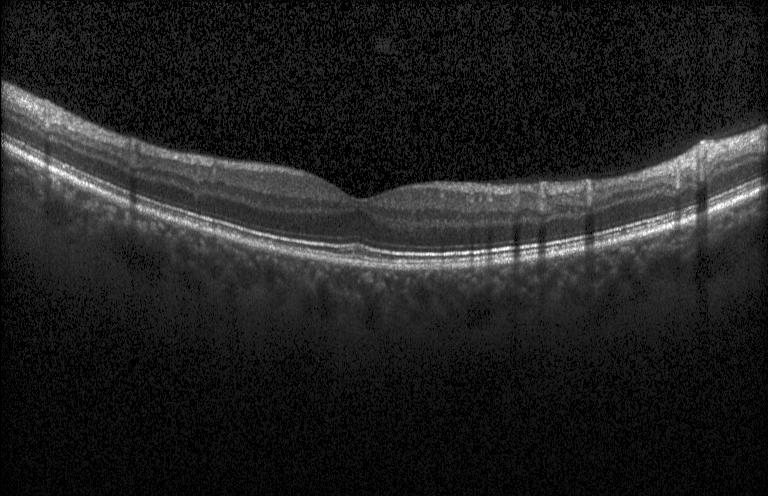
SD-OCT · OCT line scan · centered on the fovea.
Diagnosis: no evidence of choroidal neovascularization, diabetic macular edema, or drusen.